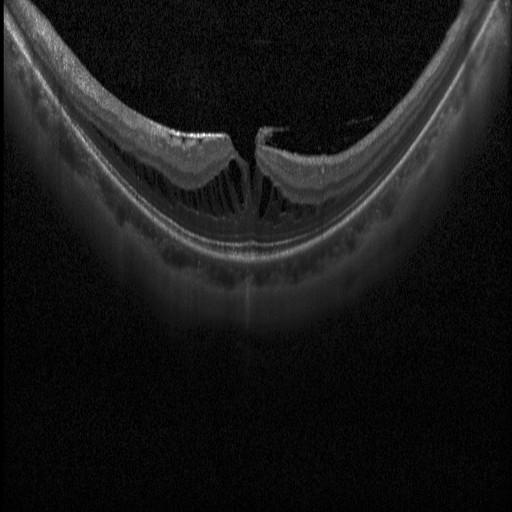 Fovea-centered. OCT line scan. SD-OCT. Impression: diabetic macular edema (DME).